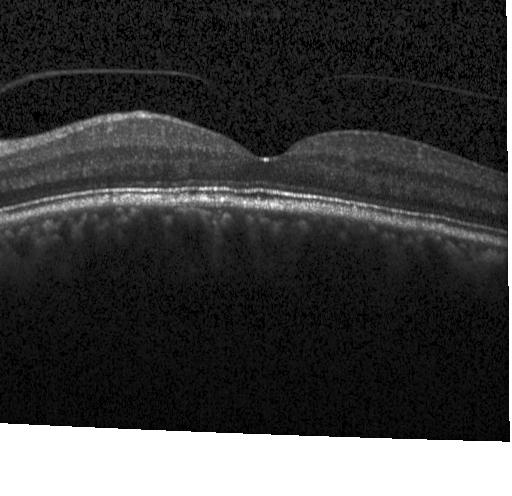 Impression: no CNV, DME, or drusen.